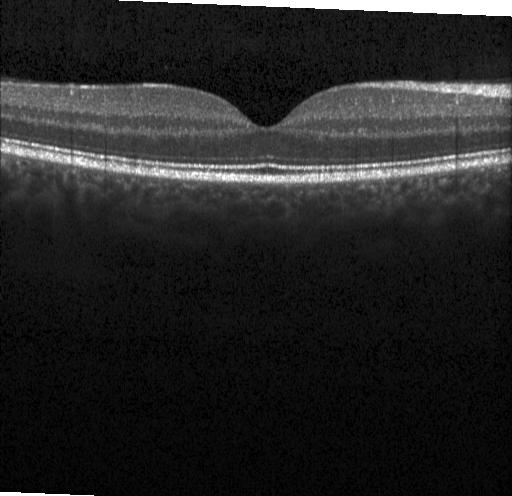 OCT B-scan, spectral-domain optical coherence tomography. No evidence of choroidal neovascularization, diabetic macular edema, or drusen.